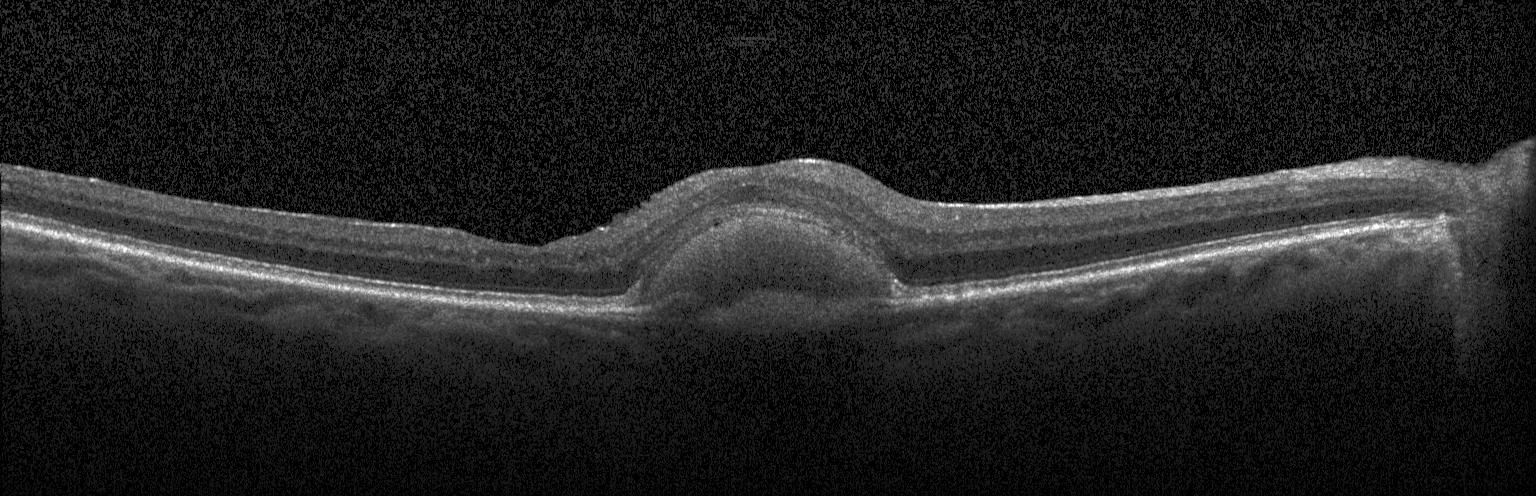

OCT finding: choroidal neovascularization.